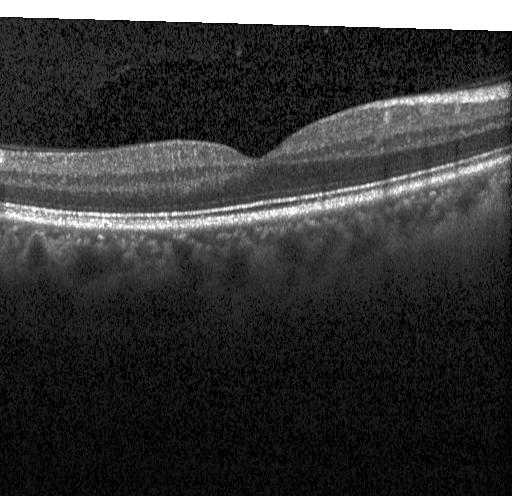

Heidelberg Spectralis. Optical coherence tomography scan
Diagnosis: no choroidal neovascularization, diabetic macular edema, or drusen.